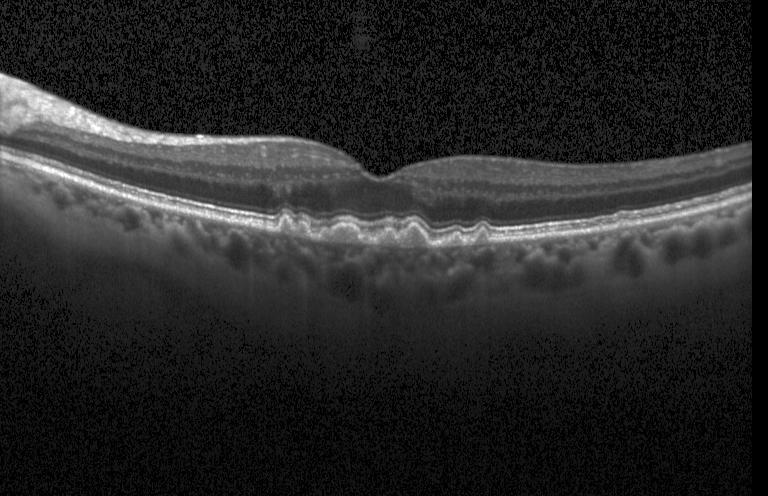 OCT B-scan showing multiple drusen.